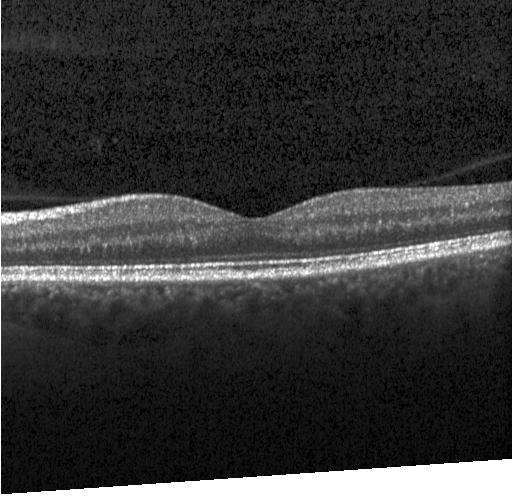

Diagnosis: no evidence of choroidal neovascularization, diabetic macular edema, or drusen.